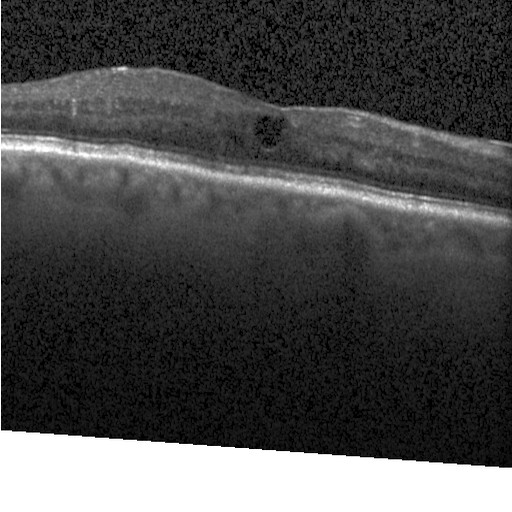 Diagnosis: diabetic macular edema (DME).